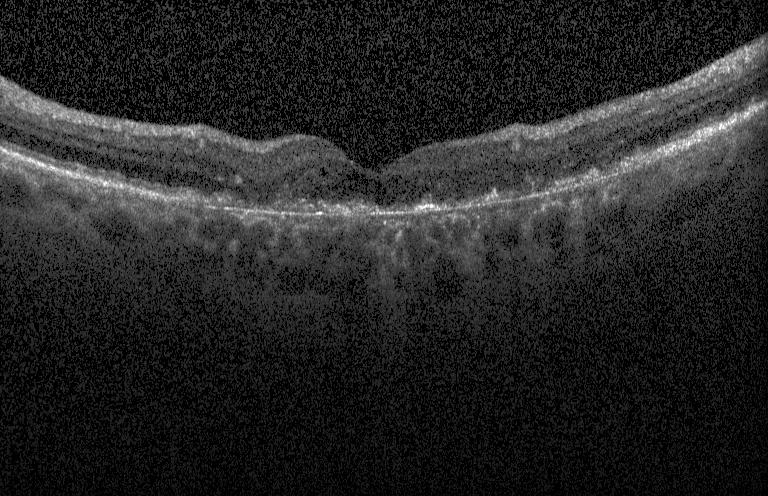

Diagnosis: a choroidal neovascular membrane.